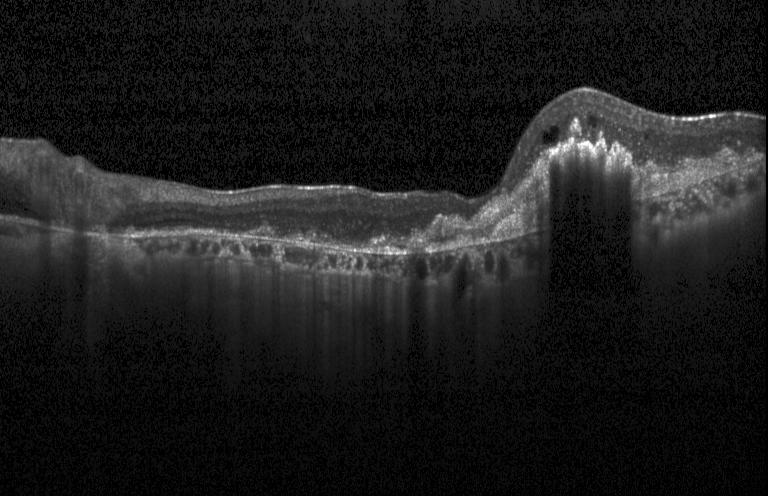
Diagnosis: CNV.